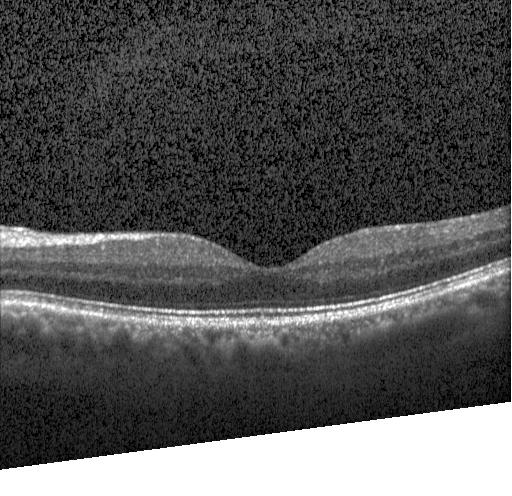
Retinal OCT B-scan. Macular scan.
Impression: no choroidal neovascularization, no diabetic macular edema, and no drusen.